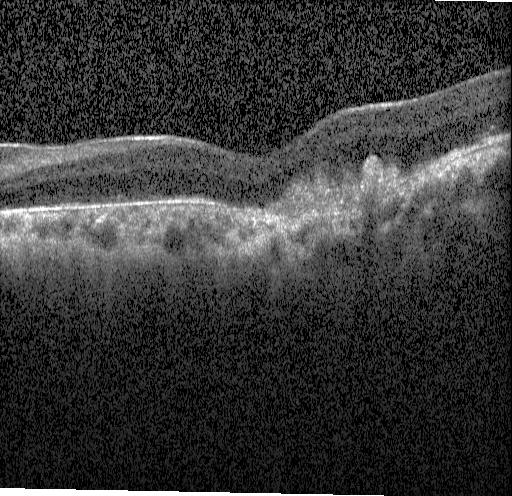 Heidelberg Spectralis OCT system · optical coherence tomography B-scan — Diagnosis: a choroidal neovascular membrane.